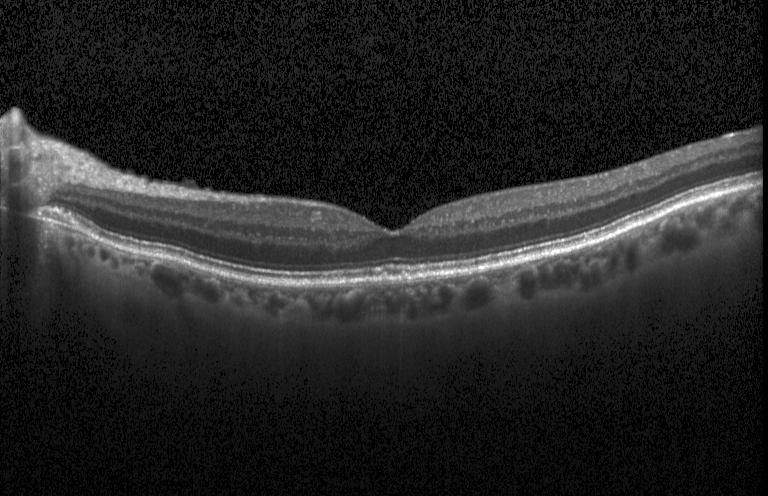
Macular scan, spectral-domain optical coherence tomography, optical coherence tomography B-scan.
Impression: no choroidal neovascularization, no diabetic macular edema, and no drusen.